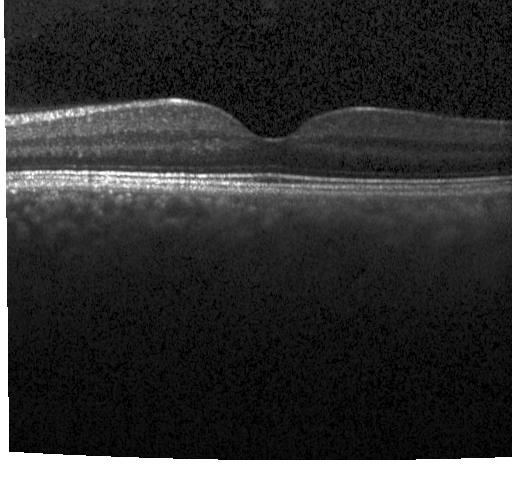
Diagnosis: no CNV, no DME, and no drusen.